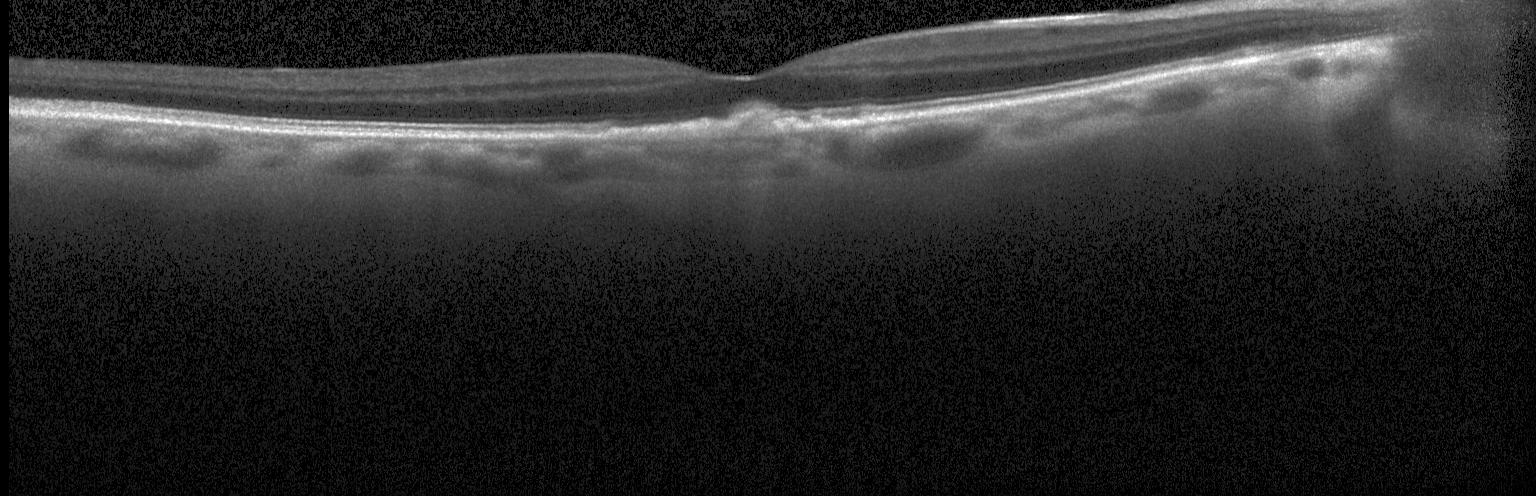
Heidelberg Spectralis OCT system. Fovea-centered. Optical coherence tomography scan. SD-OCT. This B-scan demonstrates sub-RPE drusenoid deposits.